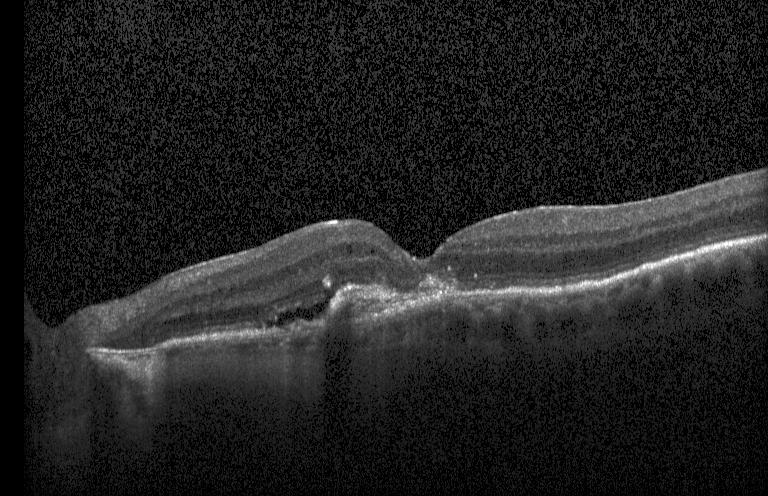
This B-scan demonstrates choroidal neovascularization (CNV).